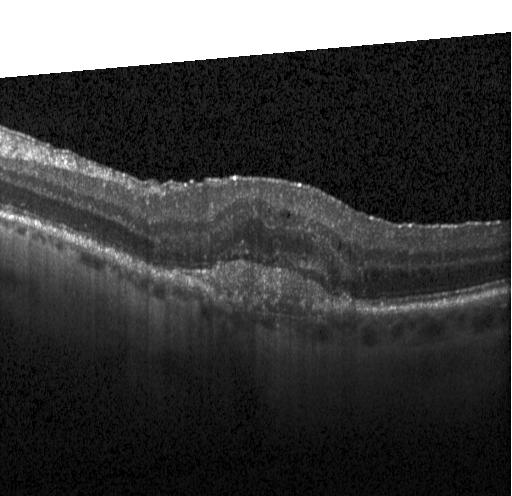 Through the macula, optical coherence tomography B-scan, spectral-domain OCT, instrument: Heidelberg Spectralis — This B-scan demonstrates a choroidal neovascular membrane.